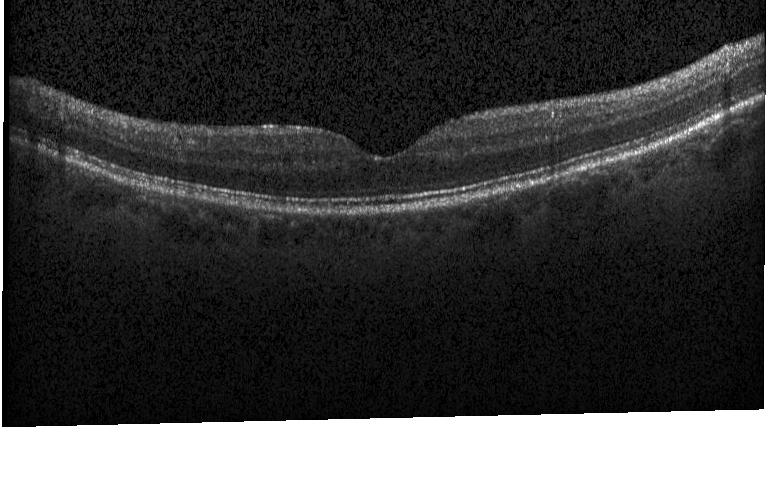 Retinal OCT B-scan, centered on the fovea, Heidelberg Spectralis OCT system — Macular OCT: no CNV, DME, or drusen.